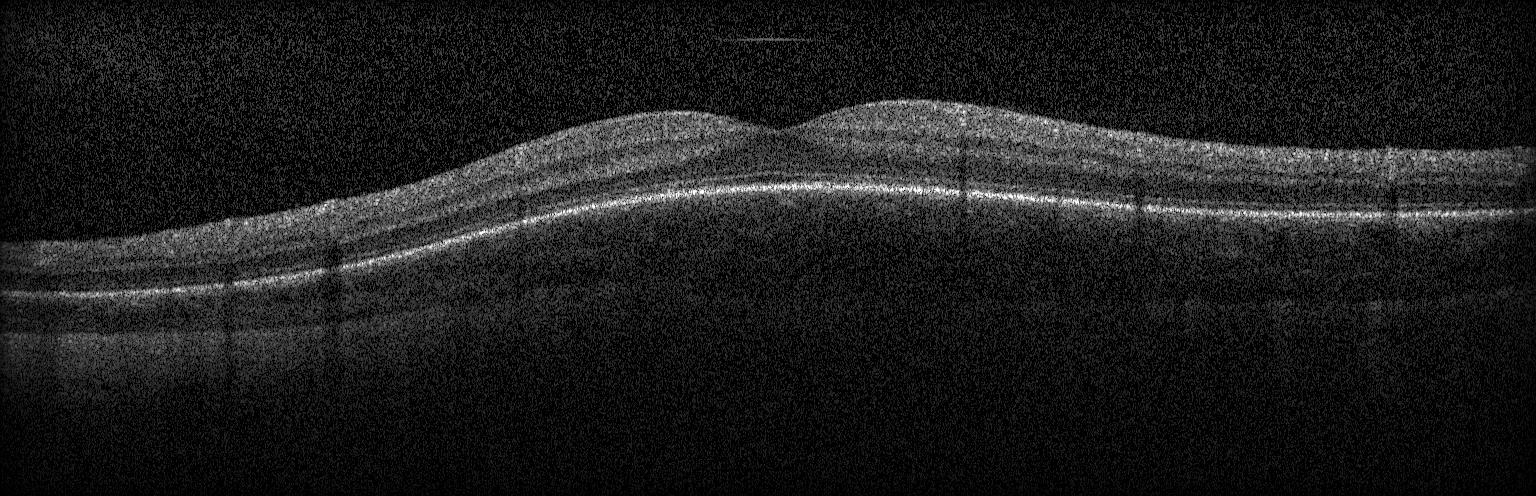 Finding: no CNV, no DME, and no drusen.